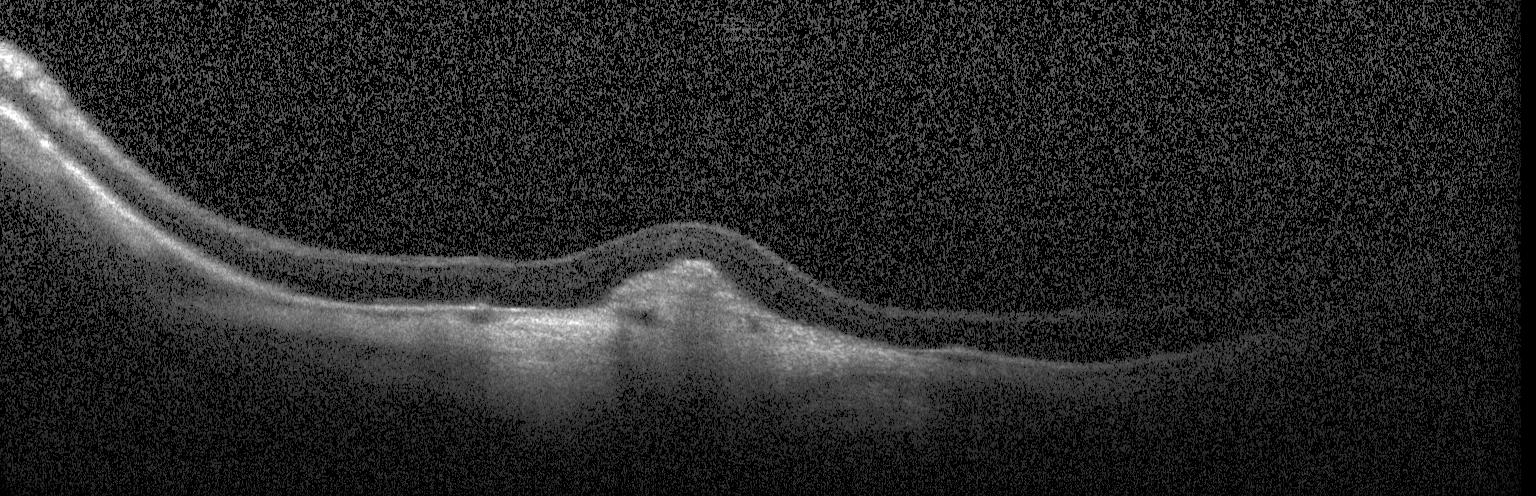

Spectral-domain optical coherence tomography · OCT line scan. Diagnosis: a choroidal neovascular membrane.